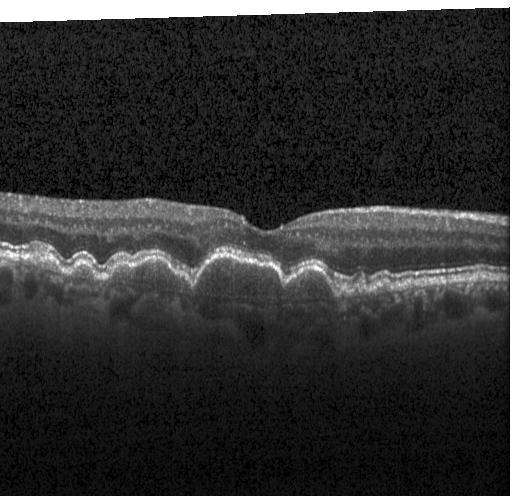
Spectral-domain OCT · centered on the fovea · acquired on a Heidelberg Spectralis · retinal OCT B-scan.
This B-scan demonstrates multiple drusen.